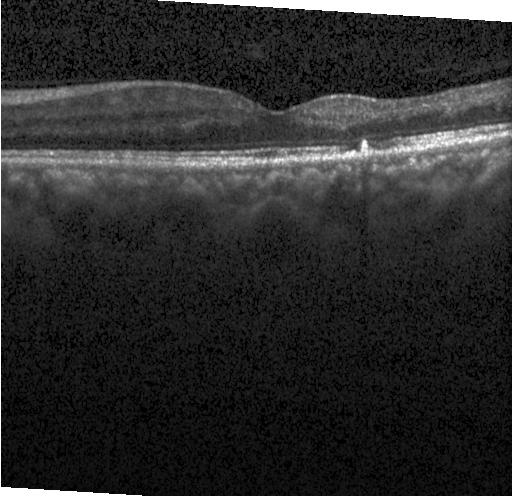 Retinal OCT B-scan. Fovea-centered. Heidelberg Spectralis. The scan shows sub-RPE drusenoid deposits.